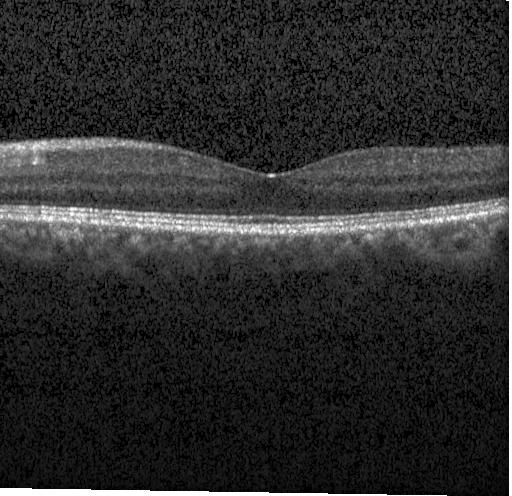 Spectral-domain optical coherence tomography. Horizontal scan through the fovea. OCT line scan — This B-scan demonstrates no choroidal neovascularization, no diabetic macular edema, and no drusen.